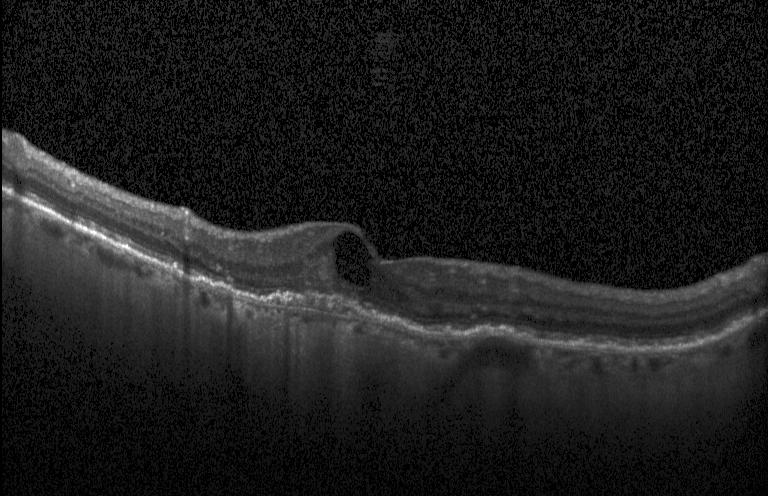 Optical coherence tomography B-scan. Instrument: Heidelberg Spectralis. Spectral-domain optical coherence tomography
Impression: choroidal neovascularization.